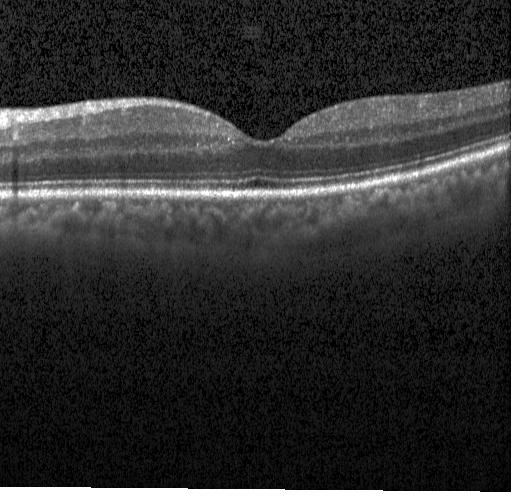
Macular OCT demonstrating neither choroidal neovascularization, diabetic macular edema, nor drusen.